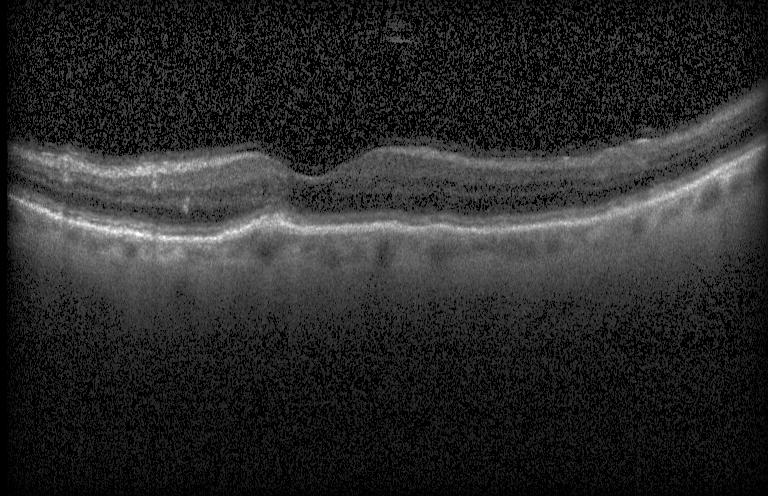
OCT line scan; spectral-domain optical coherence tomography.
Assessment: choroidal neovascularization.